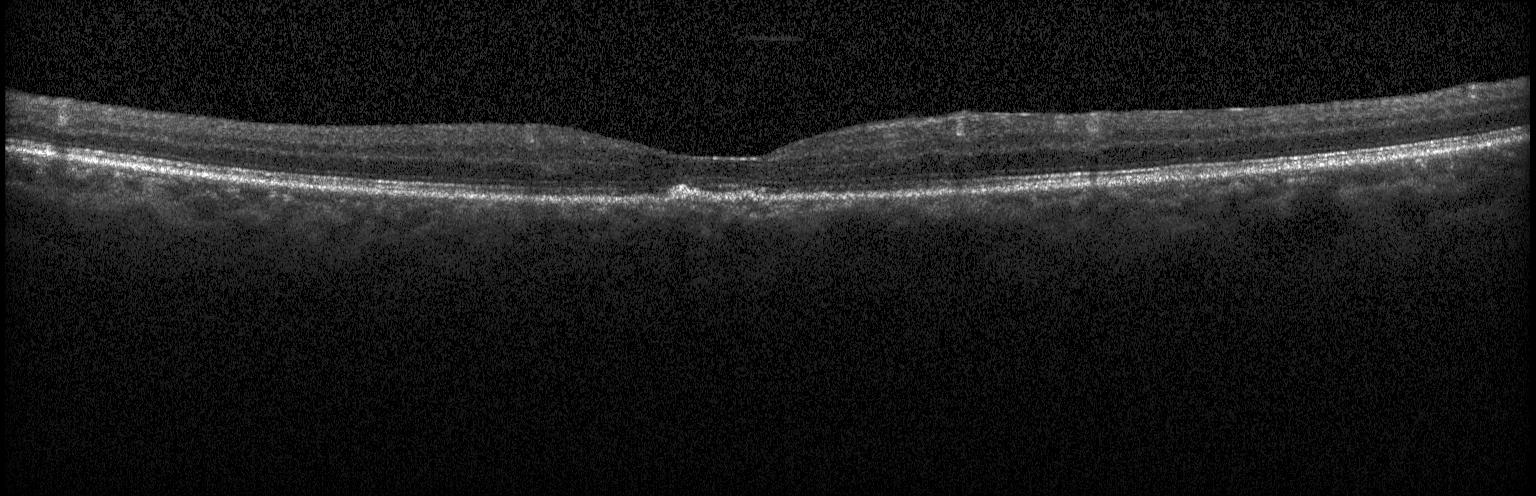
Instrument: Heidelberg Spectralis · through the macula · optical coherence tomography B-scan · spectral-domain optical coherence tomography — Finding: sub-RPE drusenoid deposits.